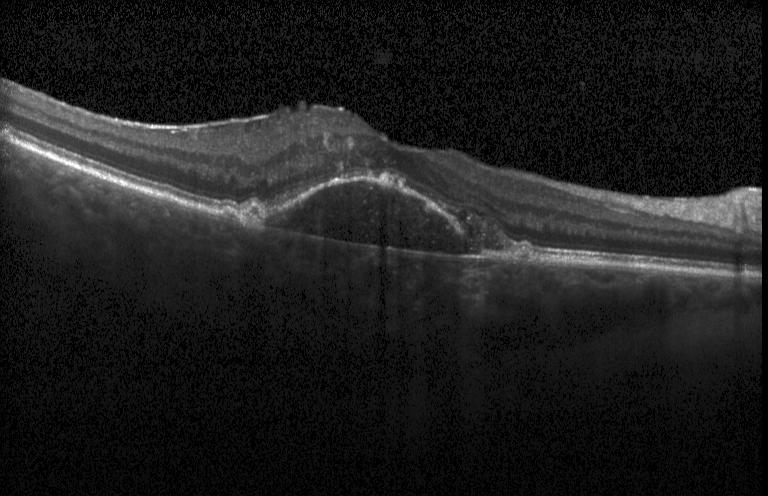 Heidelberg Spectralis OCT system; OCT B-scan. Macular OCT: choroidal neovascularization (CNV).